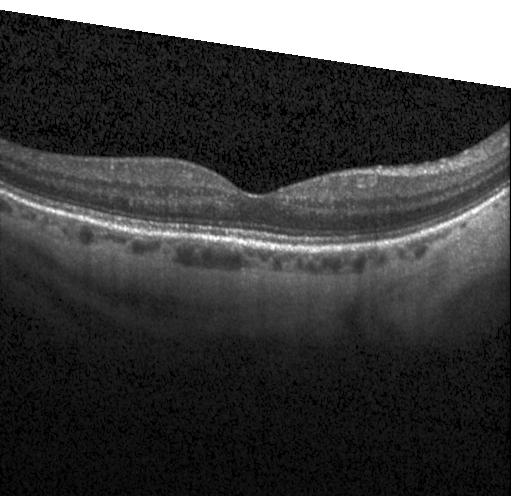
Finding: neither choroidal neovascularization, diabetic macular edema, nor drusen.